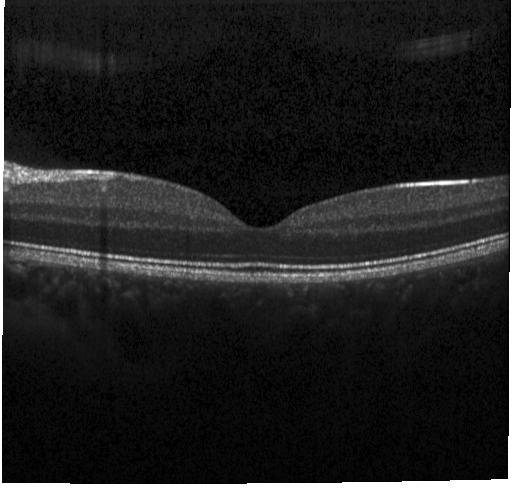
Retinal OCT cross-section; through the macula
Impression: neither choroidal neovascularization, diabetic macular edema, nor drusen.